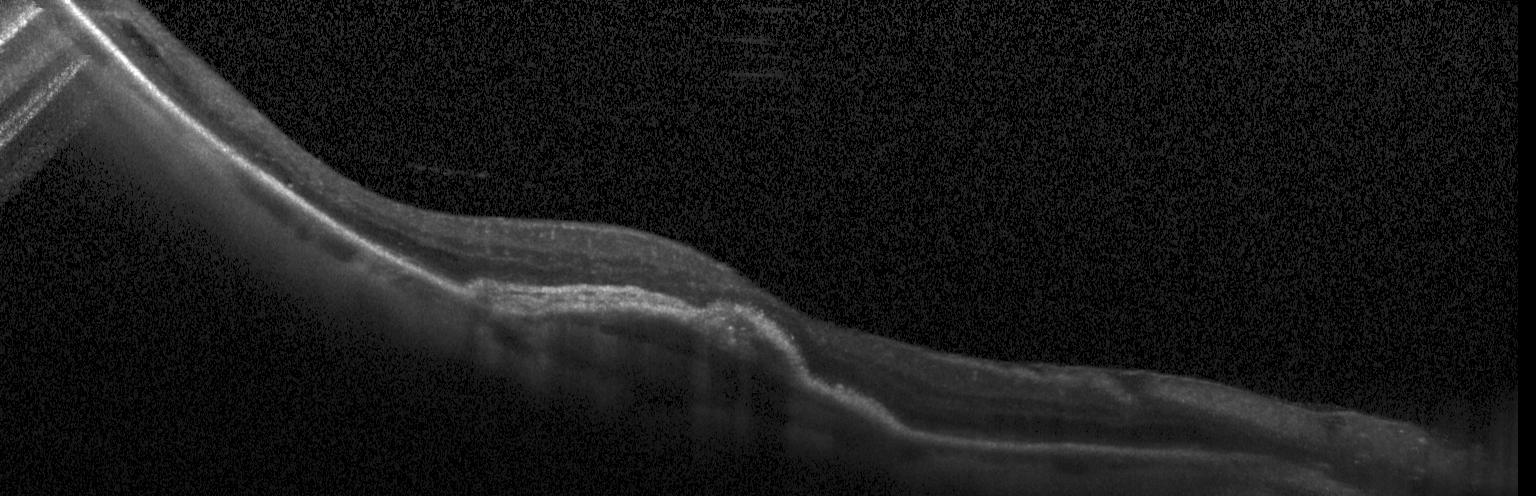 Heidelberg Spectralis; centered on the fovea; optical coherence tomography B-scan; spectral-domain optical coherence tomography — Assessment: a choroidal neovascular membrane.